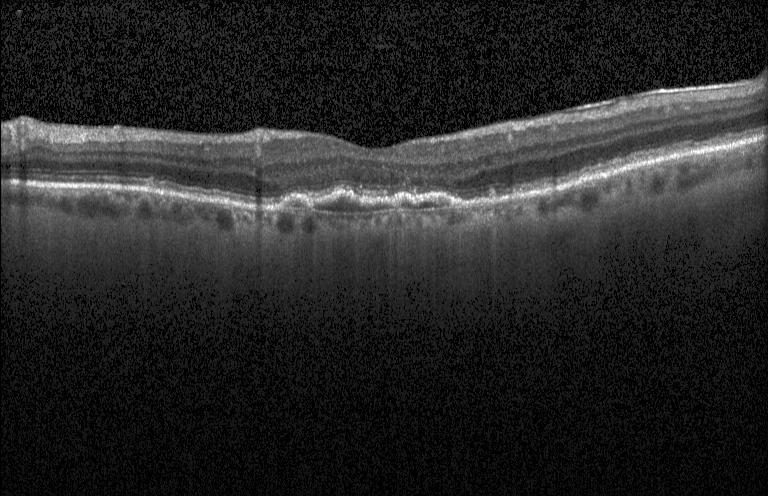

Diagnosis: a choroidal neovascular membrane.